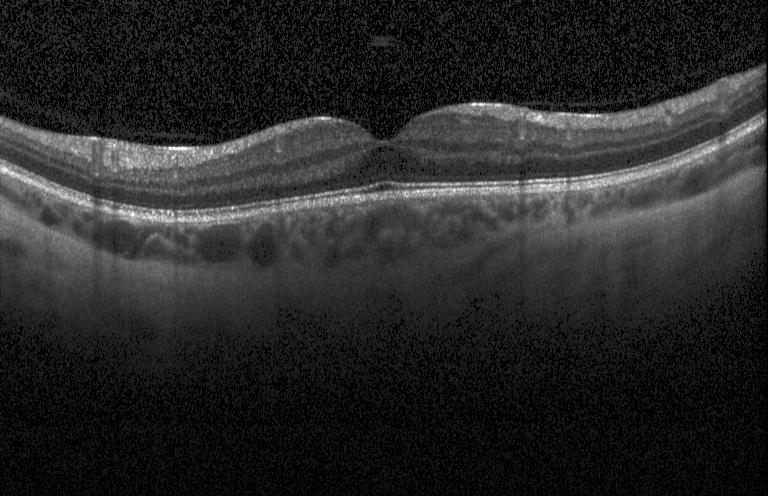 Heidelberg Spectralis OCT system; spectral-domain optical coherence tomography; OCT B-scan
Diagnosis: no evidence of choroidal neovascularization, diabetic macular edema, or drusen.